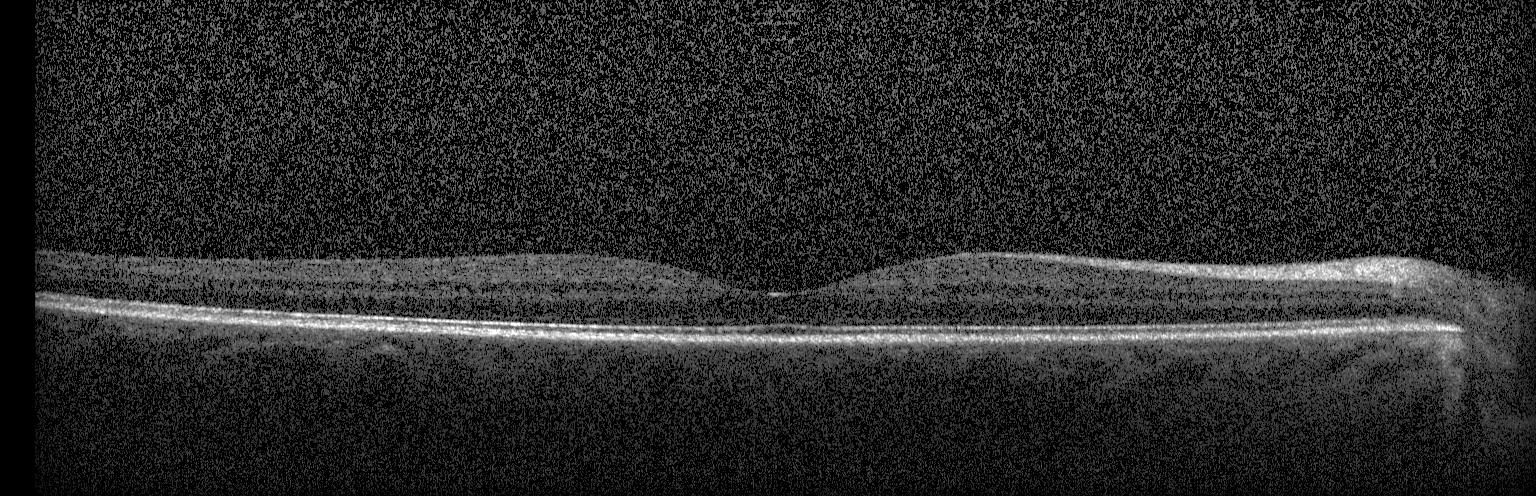 Dx: no evidence of choroidal neovascularization, diabetic macular edema, or drusen.